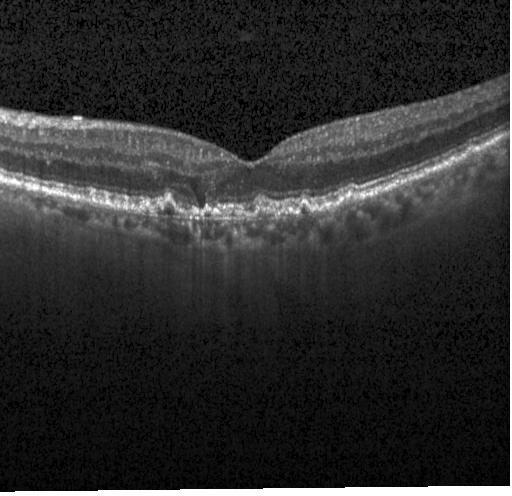 SD-OCT. Heidelberg Spectralis OCT system. Retinal OCT cross-section — Diagnosis: sub-RPE drusenoid deposits.